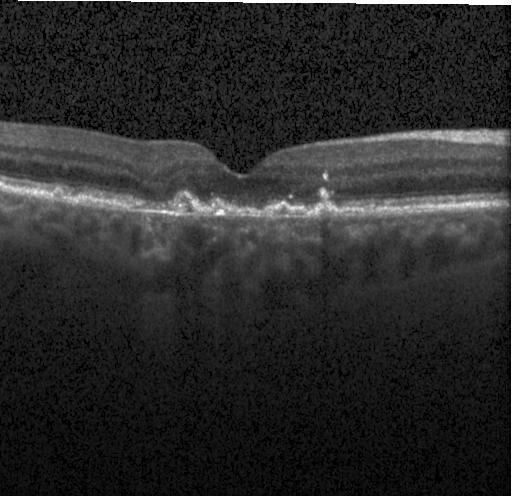
Impression: a choroidal neovascular membrane.